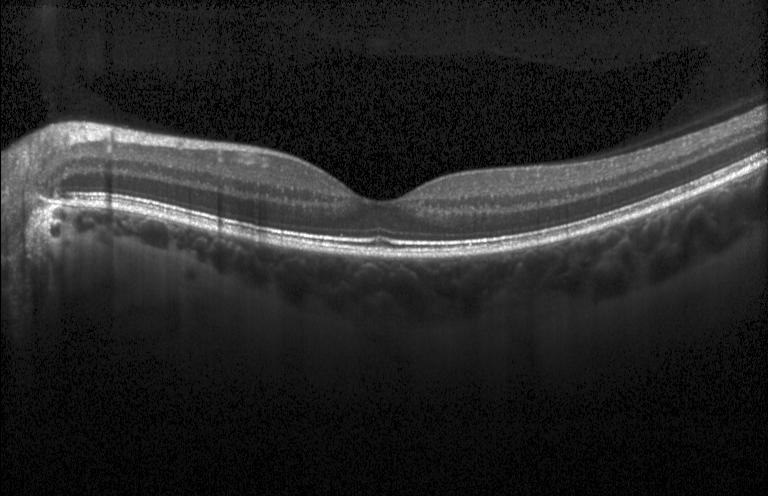 Acquired on a Heidelberg Spectralis; OCT B-scan; spectral-domain optical coherence tomography; fovea-centered — Diagnosis: no choroidal neovascularization, no diabetic macular edema, and no drusen.